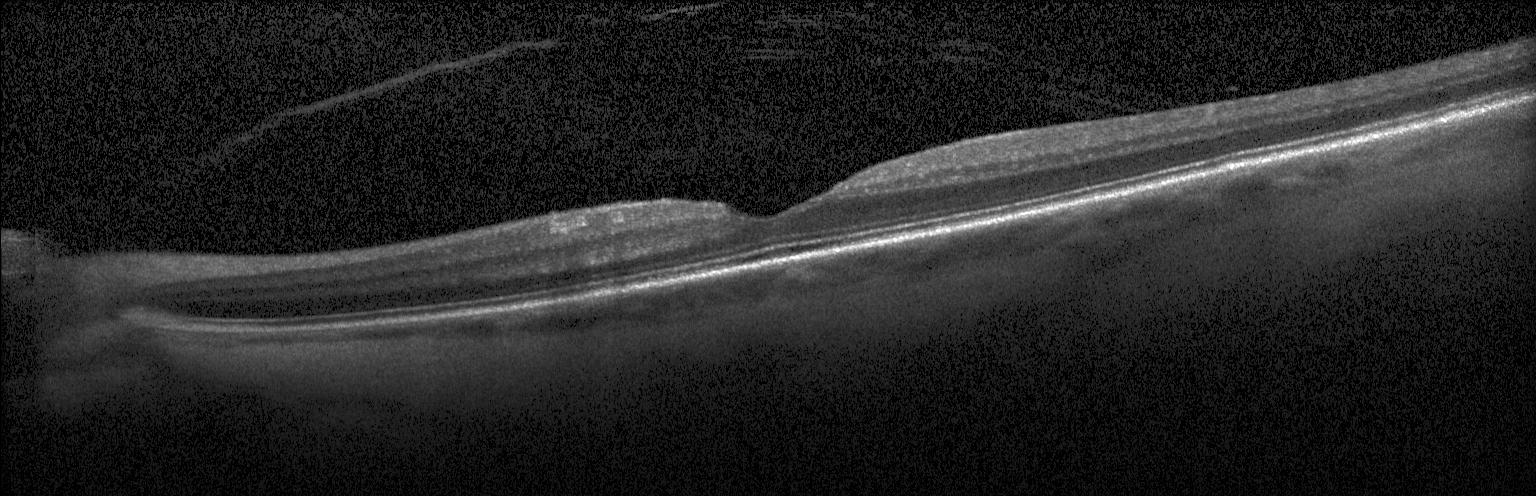

Spectral-domain OCT, horizontal scan through the fovea, optical coherence tomography B-scan. OCT finding: no evidence of choroidal neovascularization, diabetic macular edema, or drusen.